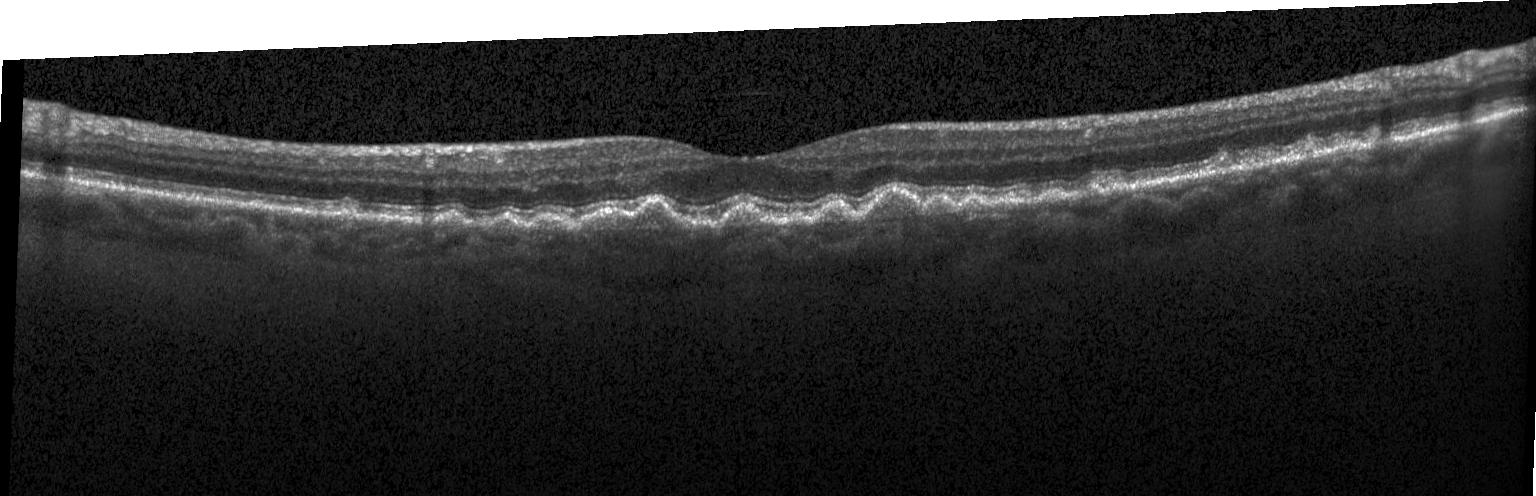

The scan shows sub-RPE drusenoid deposits.